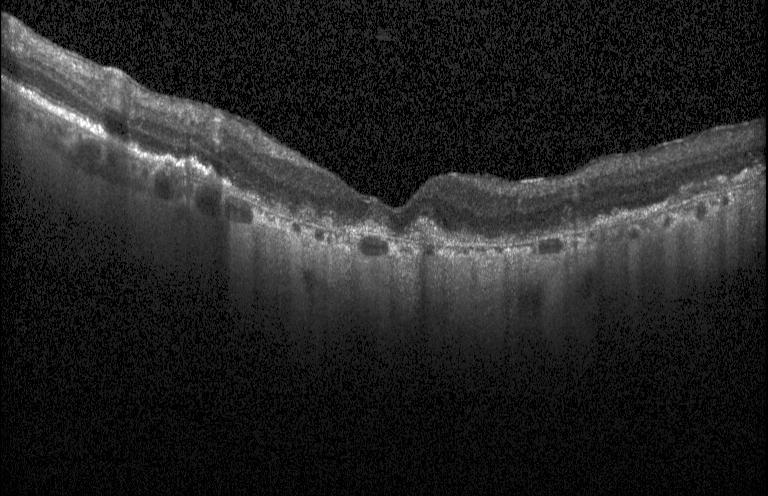

Optical coherence tomography B-scan. SD-OCT
Macular OCT: a choroidal neovascular membrane.